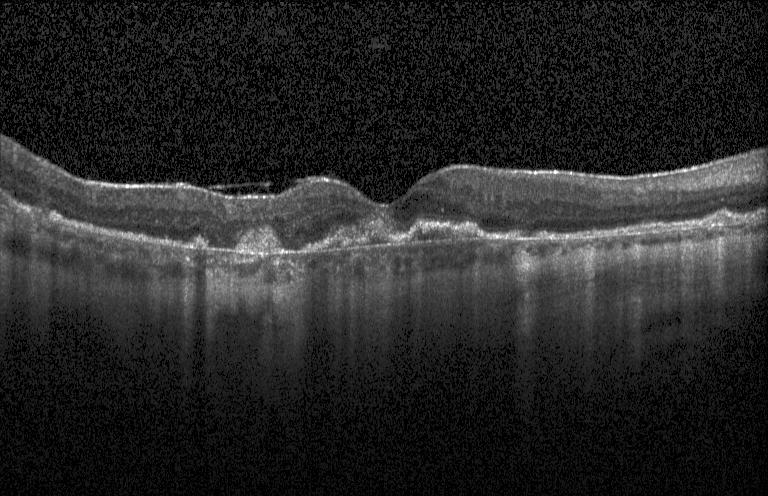 Optical coherence tomography B-scan — Finding: CNV.